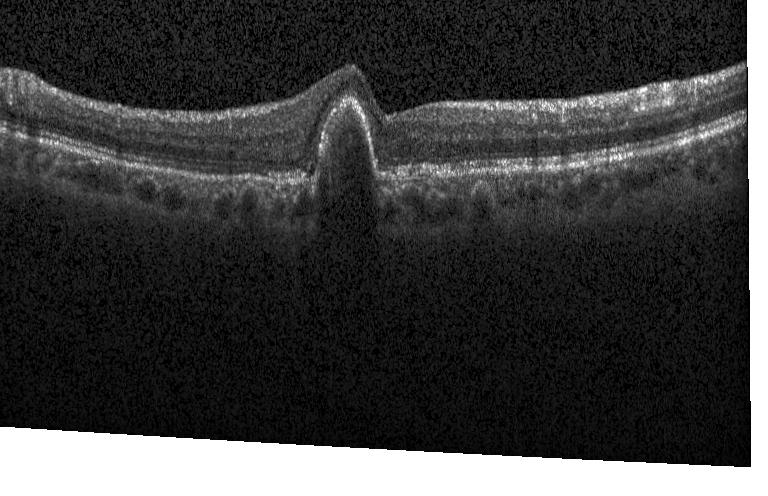 OCT scan showing CNV.